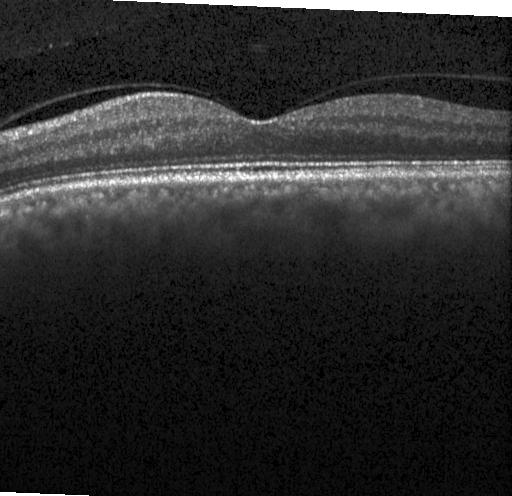

Horizontal scan through the fovea · SD-OCT · acquired on a Heidelberg Spectralis · OCT B-scan
The scan shows neither choroidal neovascularization, diabetic macular edema, nor drusen.